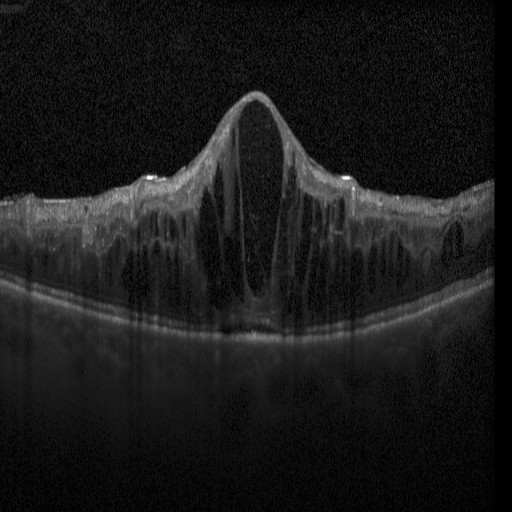 Spectral-domain OCT, optical coherence tomography B-scan, macular scan, instrument: Heidelberg Spectralis.
This B-scan demonstrates diabetic macular edema (DME).